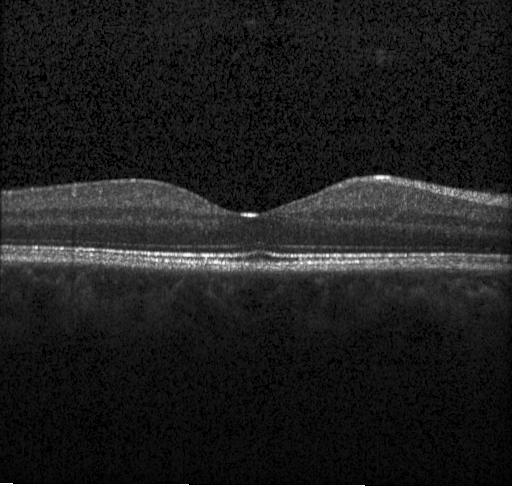
Optical coherence tomography scan, macular scan, Heidelberg Spectralis OCT system, spectral-domain OCT
Assessment: no evidence of choroidal neovascularization, diabetic macular edema, or drusen.